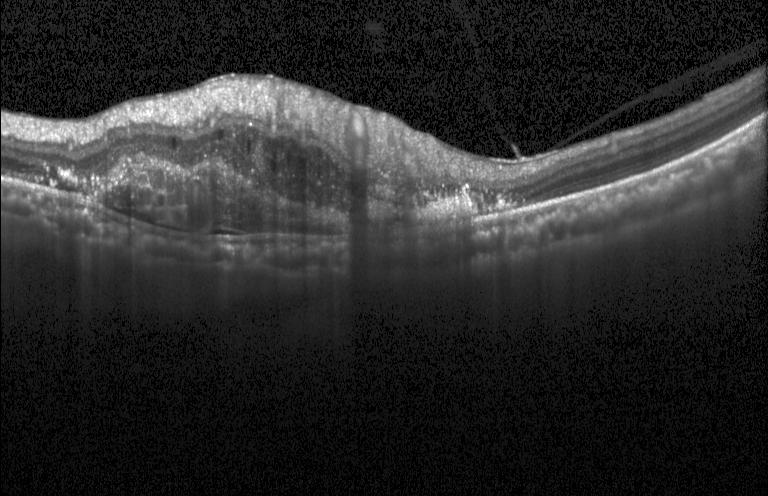

Optical coherence tomography B-scan, through the macula.
This B-scan demonstrates a choroidal neovascular membrane.